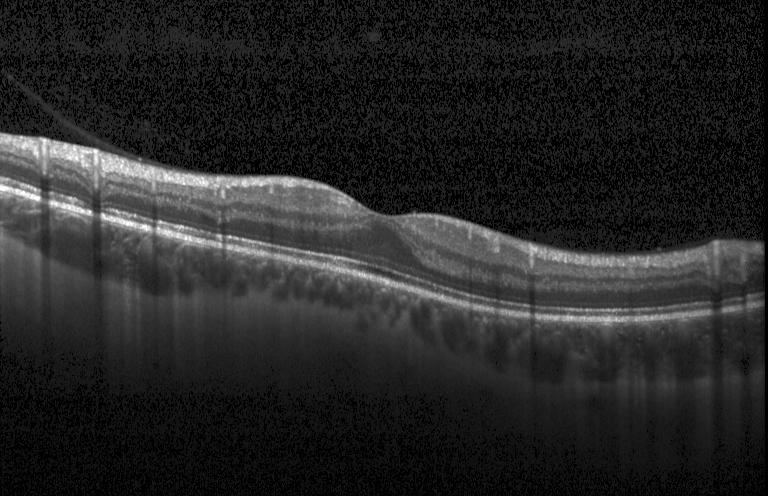
Assessment: neither choroidal neovascularization, diabetic macular edema, nor drusen.